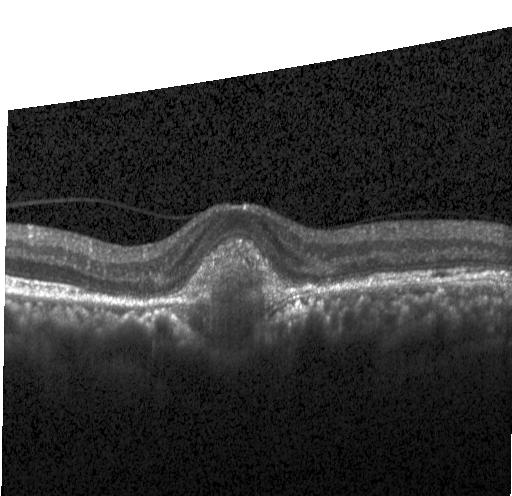

Macular OCT: choroidal neovascularization.